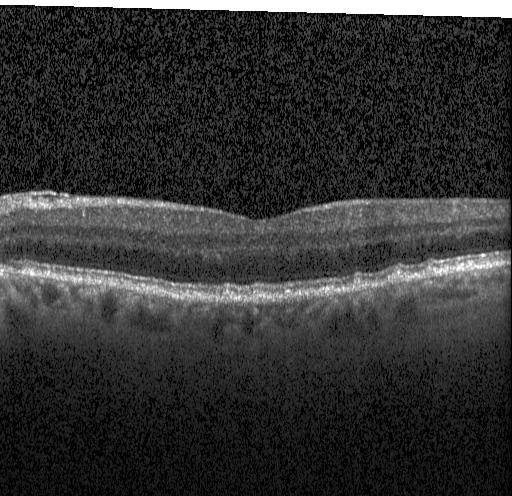 OCT finding: sub-RPE drusenoid deposits.